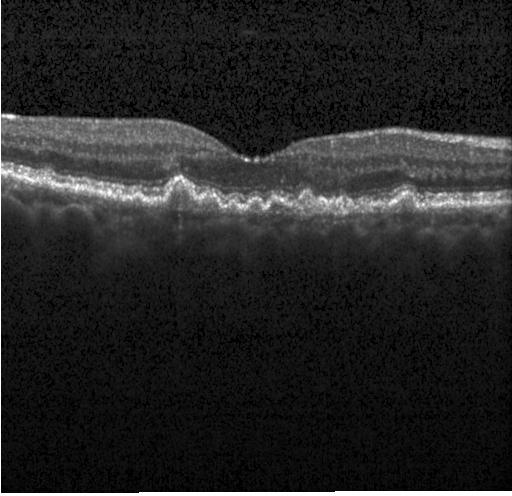
Retinal OCT cross-section, through the macula, spectral-domain optical coherence tomography.
Impression: drusen.